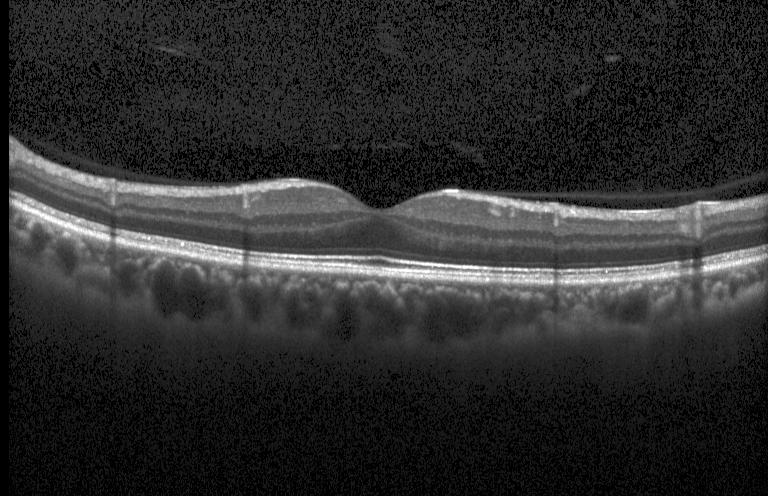
Spectral-domain optical coherence tomography; retinal OCT cross-section — Dx: no choroidal neovascularization, diabetic macular edema, or drusen.